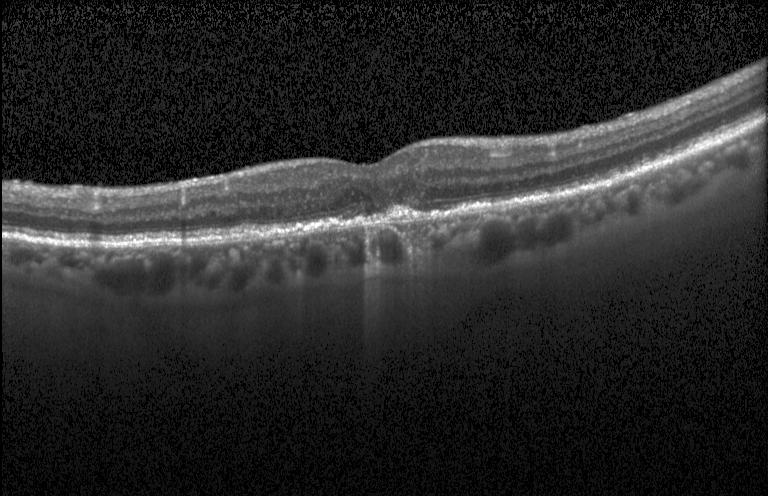

OCT finding: a choroidal neovascular membrane.